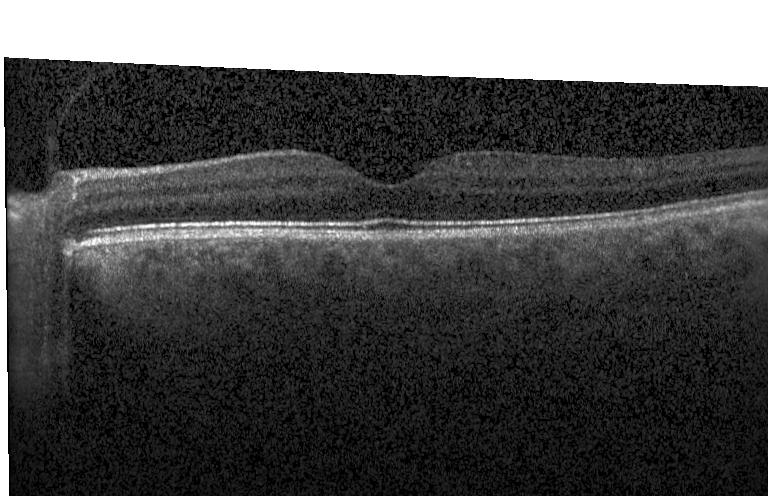

Fovea-centered · retinal OCT cross-section · spectral-domain optical coherence tomography · acquired on a Heidelberg Spectralis.
Assessment: neither choroidal neovascularization, diabetic macular edema, nor drusen.